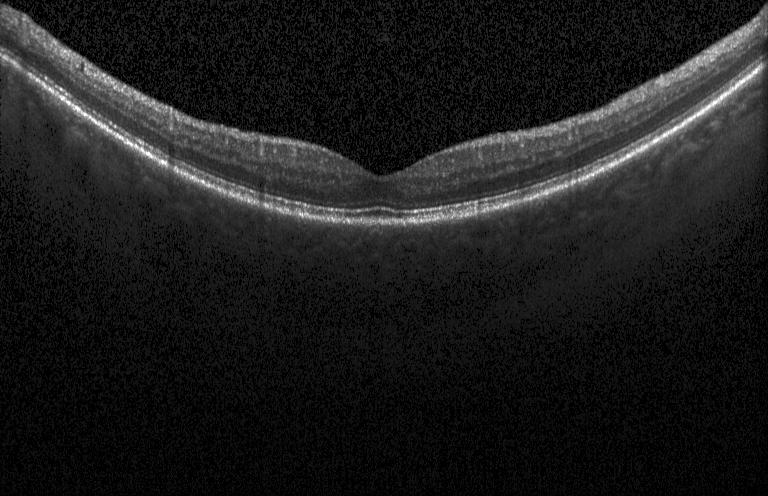 Finding: neither CNV, DME, nor drusen.